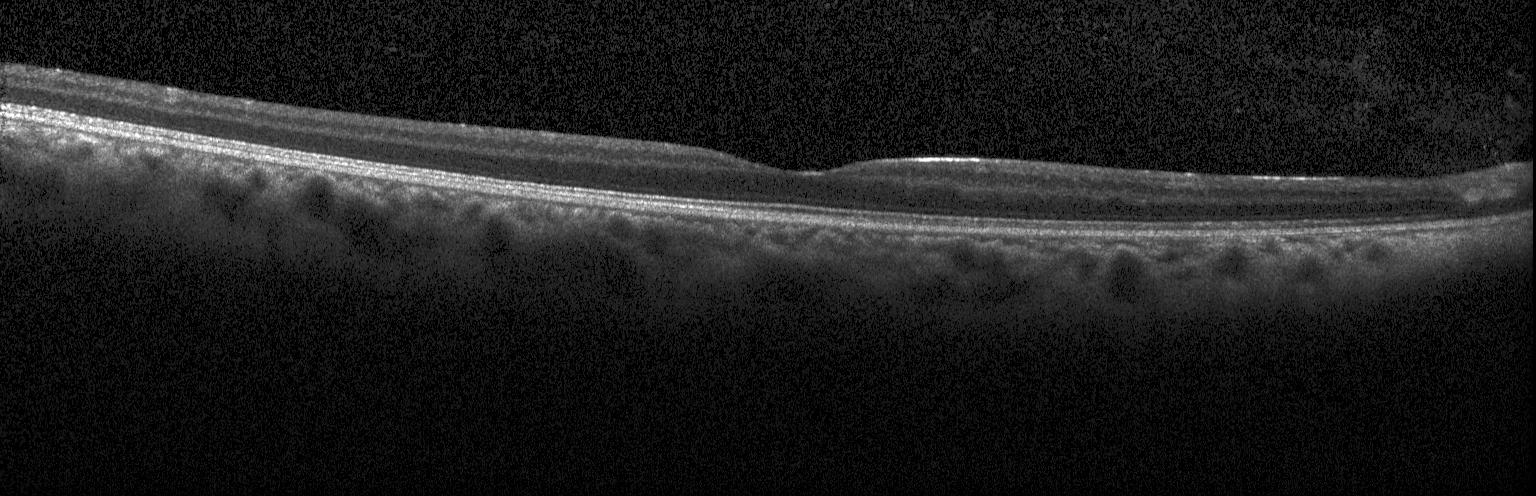
Macular OCT: no evidence of choroidal neovascularization, diabetic macular edema, or drusen.